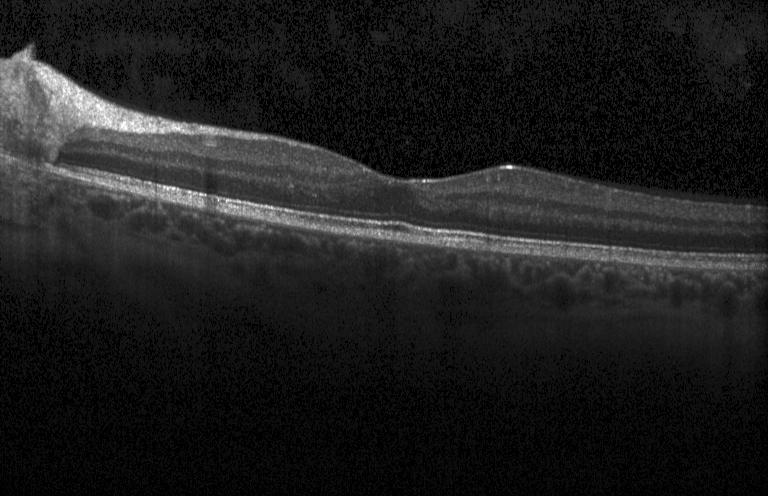 Impression: no CNV, DME, or drusen.